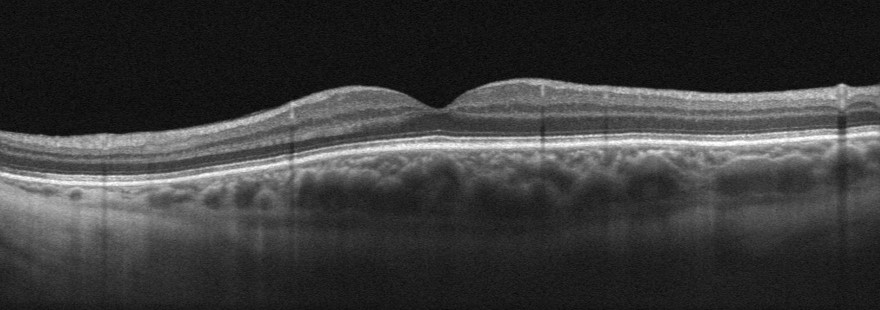
Optical coherence tomography B-scan; Optovue Avanti RTVue XR; fovea-centered.
Absence of AMD, DME, ERM, RAO, RVO, and vitreomacular interface disease.